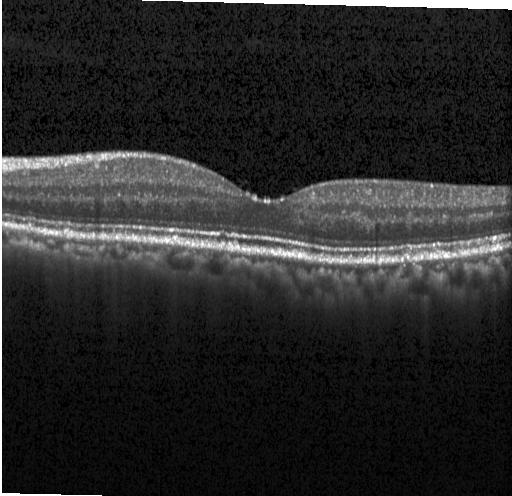

Optical coherence tomography scan, spectral-domain OCT — OCT finding: no evidence of choroidal neovascularization, diabetic macular edema, or drusen.